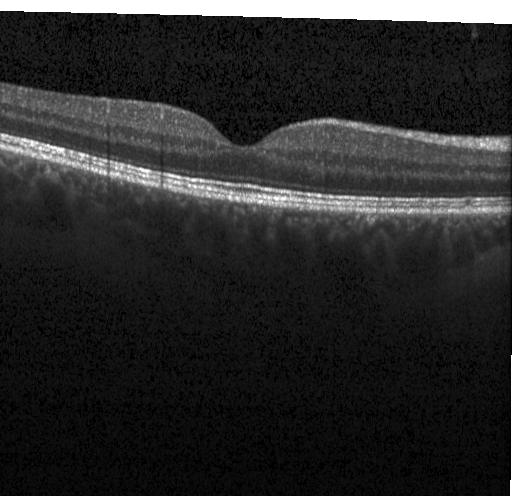

SD-OCT; OCT line scan. Impression: neither CNV, DME, nor drusen.